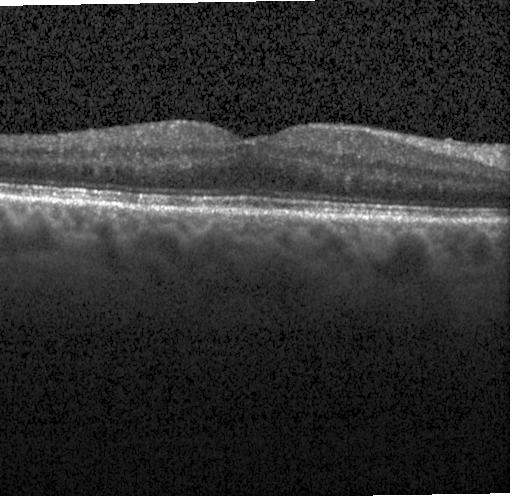
Acquired on a Heidelberg Spectralis, spectral-domain OCT, optical coherence tomography B-scan, fovea-centered
OCT finding: no evidence of choroidal neovascularization, diabetic macular edema, or drusen.